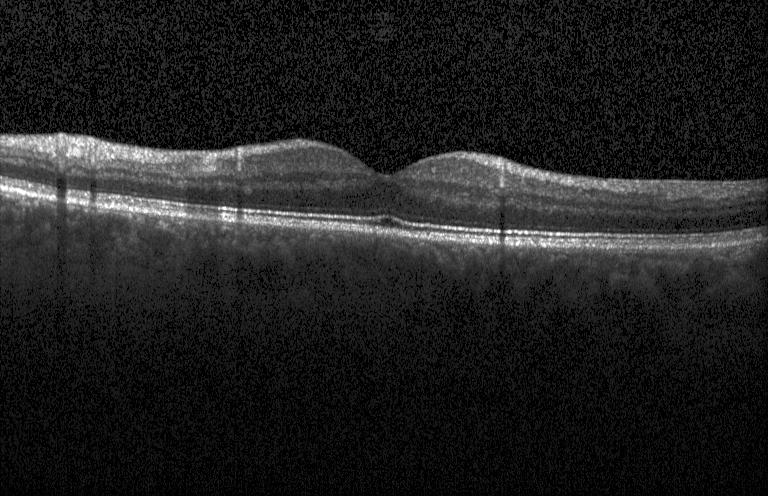 Optical coherence tomography scan — Finding: no evidence of CNV, DME, or drusen.